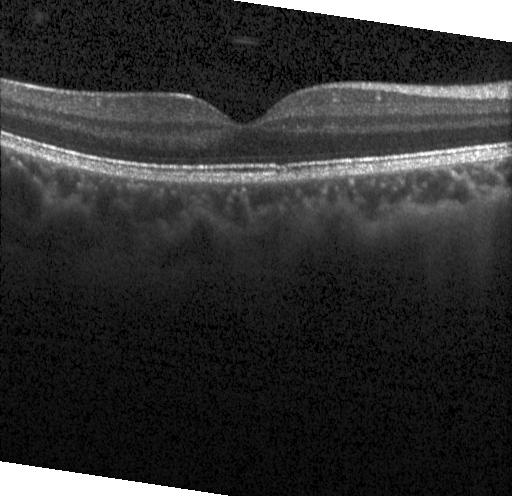
The scan shows no choroidal neovascularization, no diabetic macular edema, and no drusen.